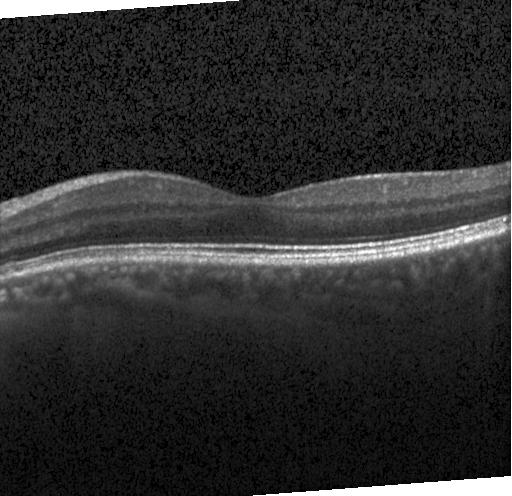 Finding: no CNV, no DME, and no drusen.